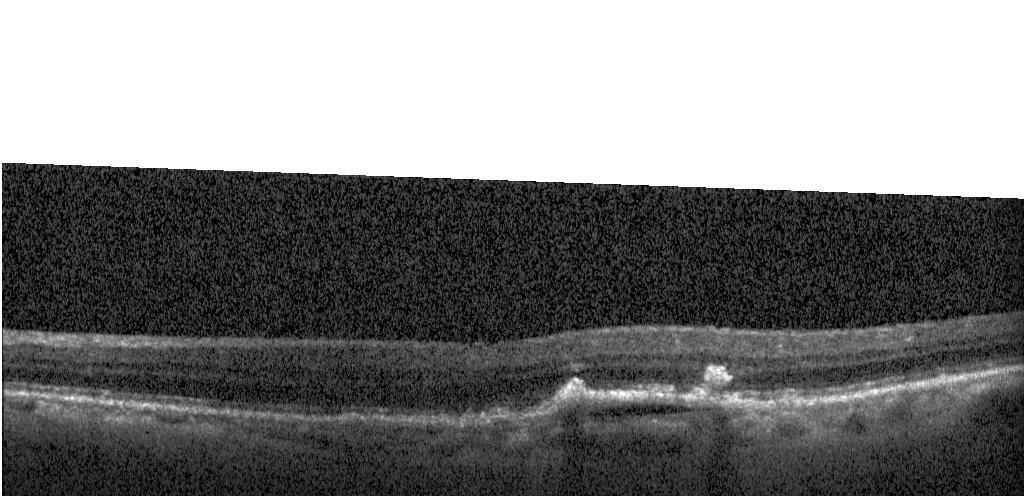
Heidelberg Spectralis OCT system, spectral-domain OCT, retinal OCT cross-section, through the macula.
Assessment: choroidal neovascularization (CNV).